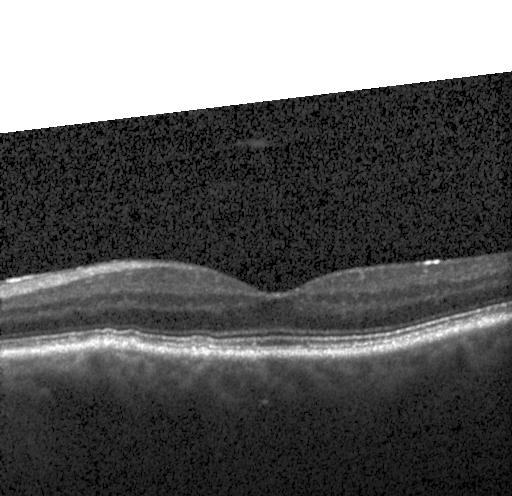

Assessment: drusen.